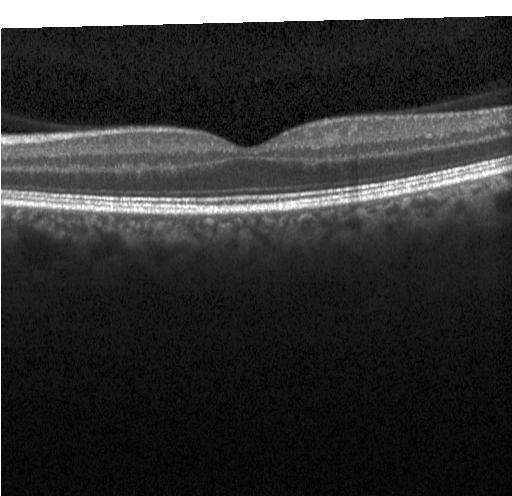
Optical coherence tomography B-scan. Impression: no choroidal neovascularization, diabetic macular edema, or drusen.